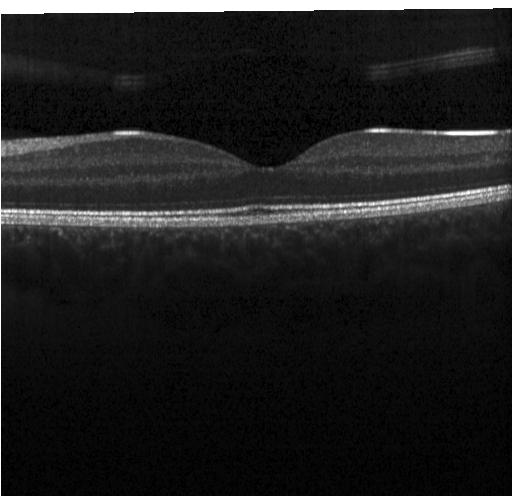
OCT scan showing neither choroidal neovascularization, diabetic macular edema, nor drusen.